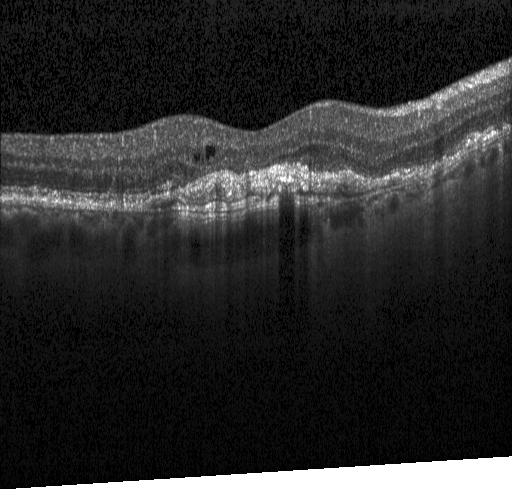 Impression: a choroidal neovascular membrane.